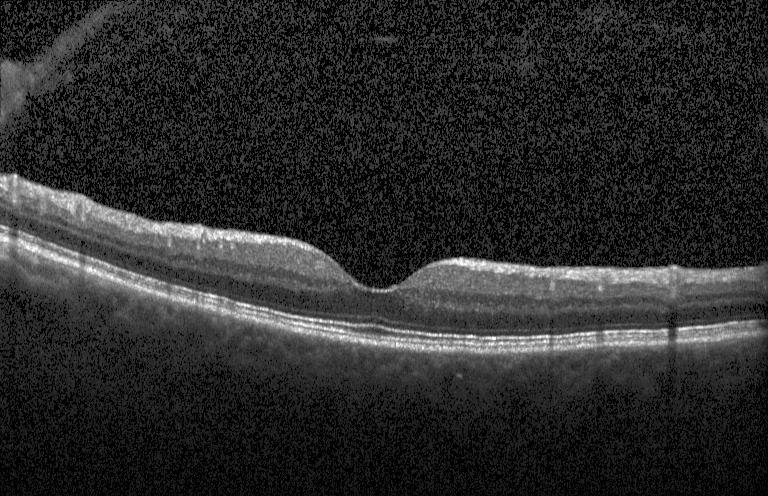

The scan shows no CNV, DME, or drusen.